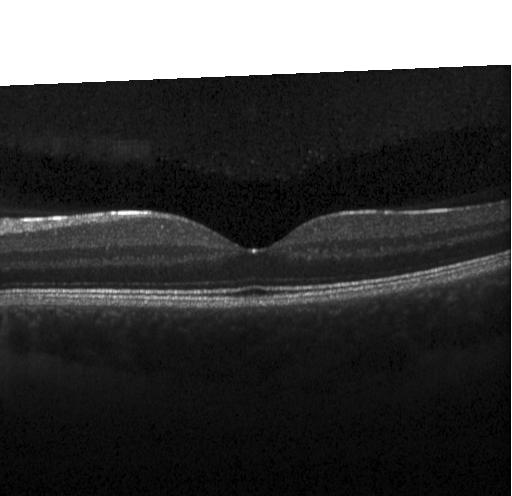
Spectral-domain OCT; optical coherence tomography scan.
Dx: no choroidal neovascularization, no diabetic macular edema, and no drusen.